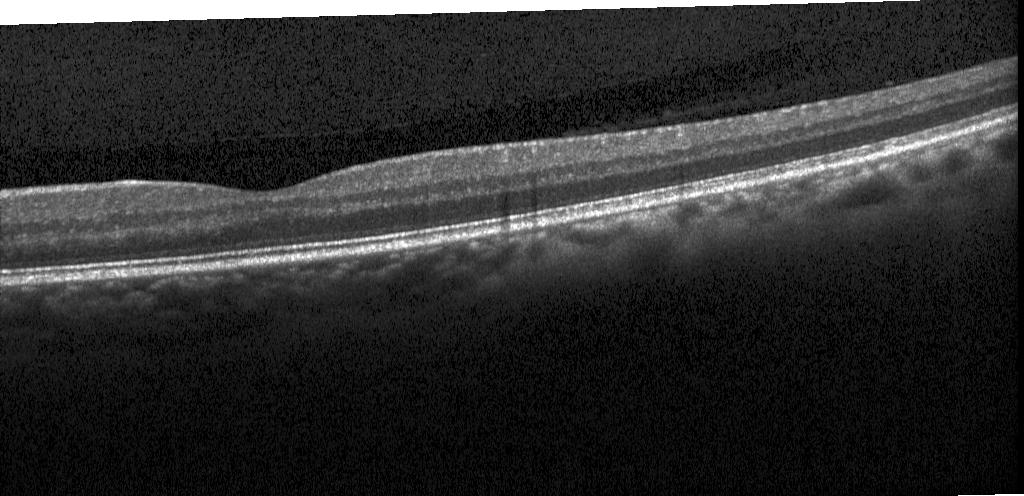 Retinal OCT cross-section, acquired on a Heidelberg Spectralis, SD-OCT. No choroidal neovascularization, no diabetic macular edema, and no drusen.